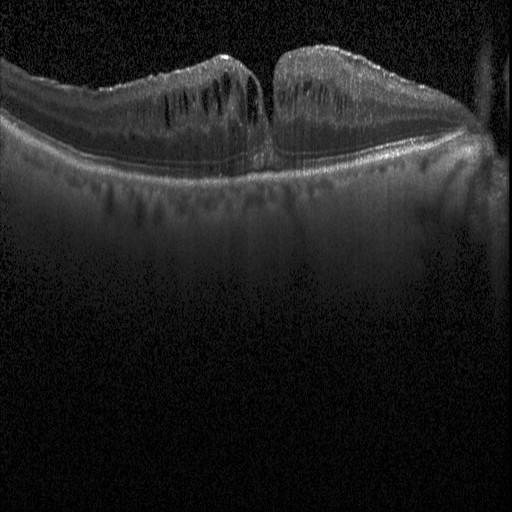 OCT line scan; spectral-domain OCT — Impression: diabetic macular edema.